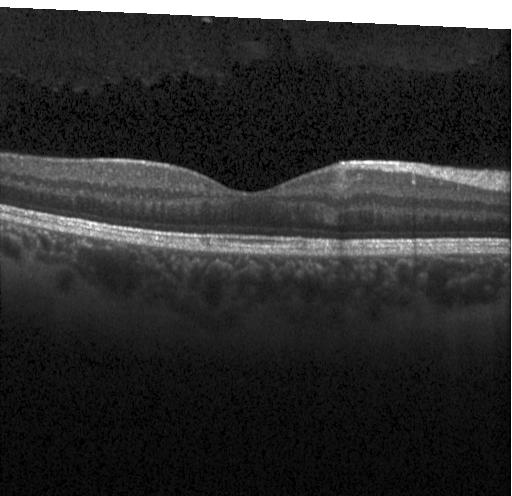
OCT scan showing no evidence of choroidal neovascularization, diabetic macular edema, or drusen.